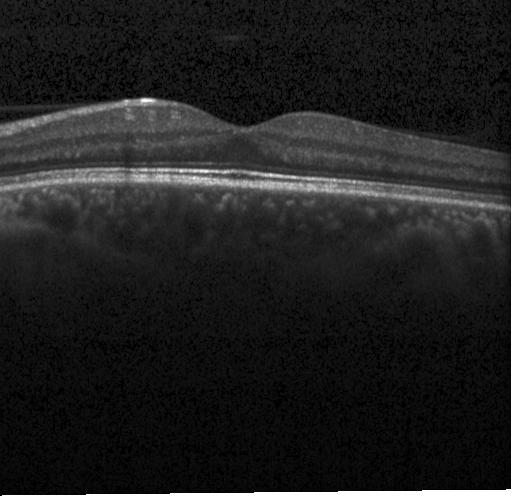

Diagnosis: neither choroidal neovascularization, diabetic macular edema, nor drusen.